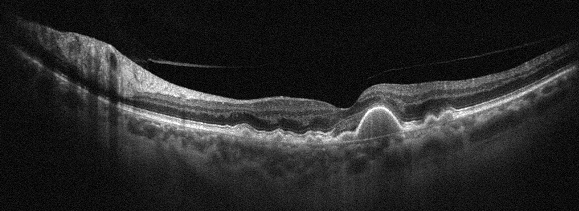

Through the macula. Retinal OCT B-scan. Optovue Avanti RTVue XR.
Dx: AMD.